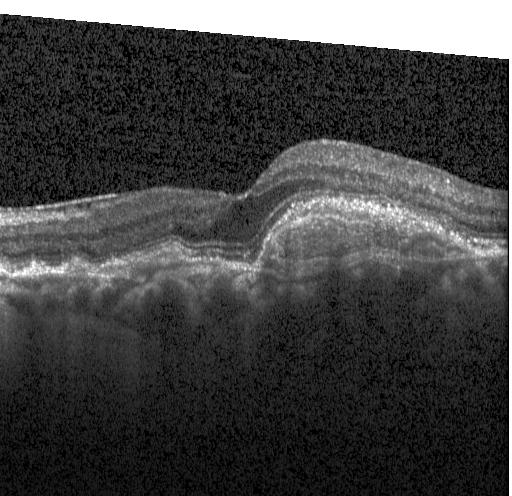
Retinal OCT B-scan
Choroidal neovascularization.